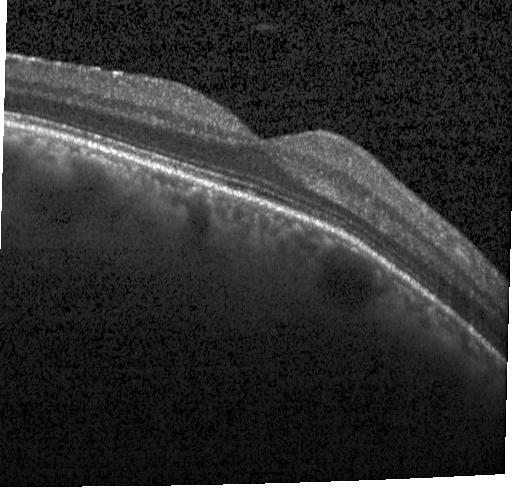 OCT B-scan. This B-scan demonstrates no choroidal neovascularization, no diabetic macular edema, and no drusen.